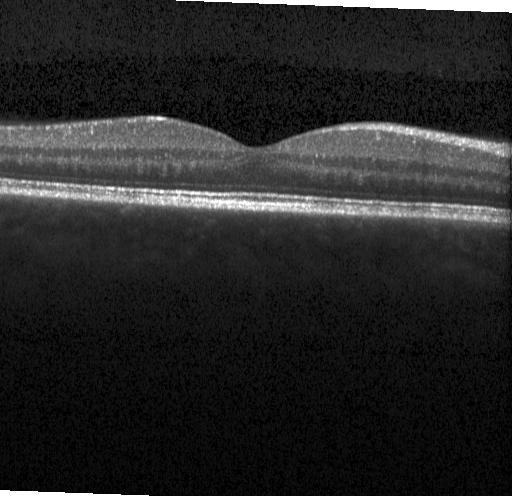
Dx: no evidence of CNV, DME, or drusen.